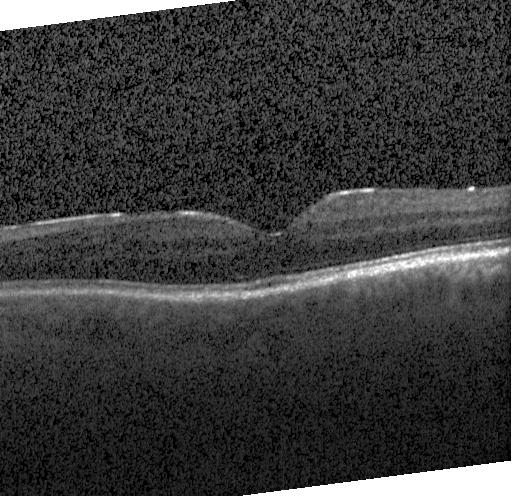
Impression: neither choroidal neovascularization, diabetic macular edema, nor drusen.